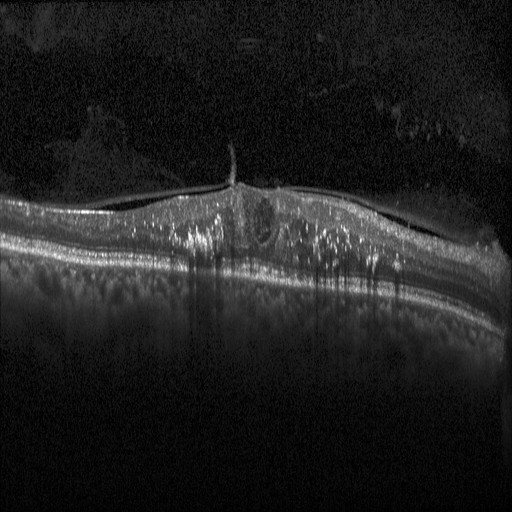 Retinal OCT cross-section — Diagnosis: DME.